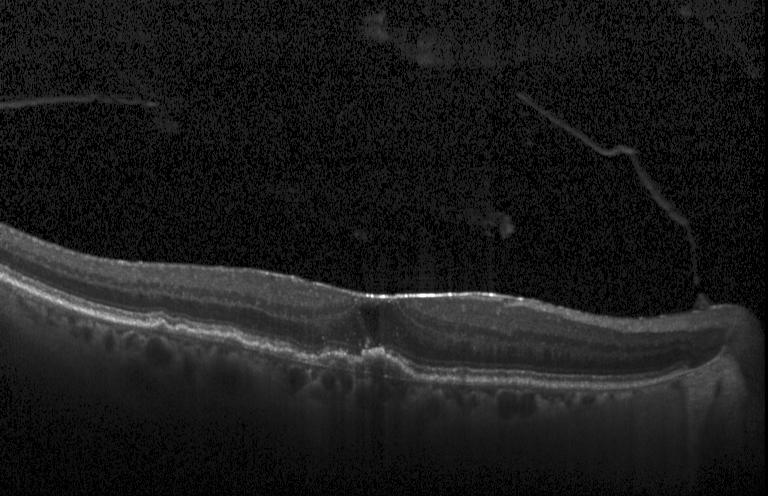
Centered on the fovea · instrument: Heidelberg Spectralis · spectral-domain optical coherence tomography · OCT line scan. Finding: CNV.